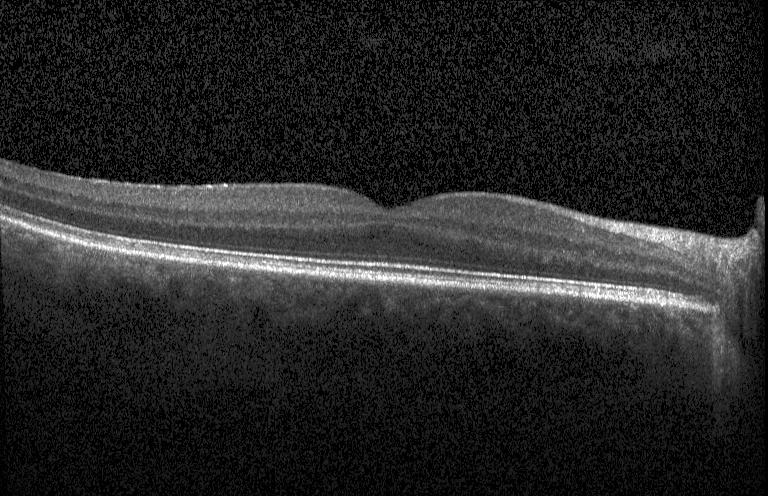 Retinal OCT cross-section
This B-scan demonstrates neither choroidal neovascularization, diabetic macular edema, nor drusen.